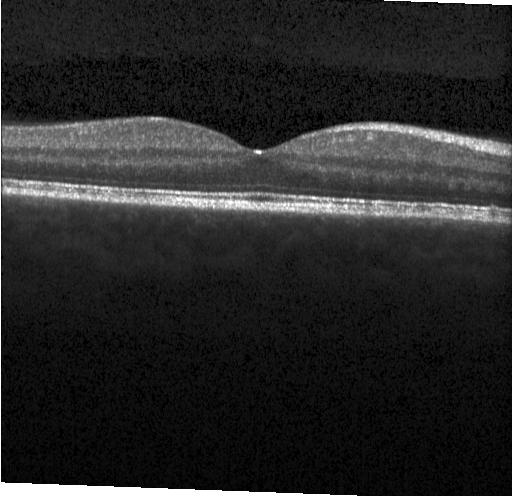
Macular OCT demonstrating no evidence of choroidal neovascularization, diabetic macular edema, or drusen.